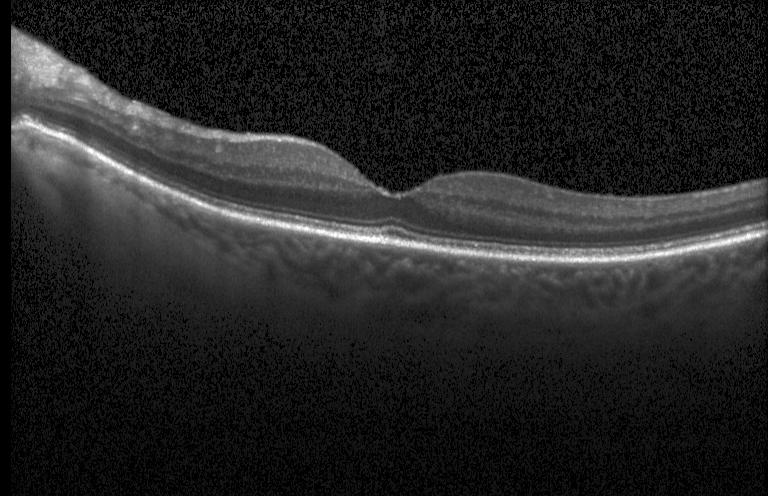 Retinal OCT cross-section, through the macula
Finding: no evidence of CNV, DME, or drusen.